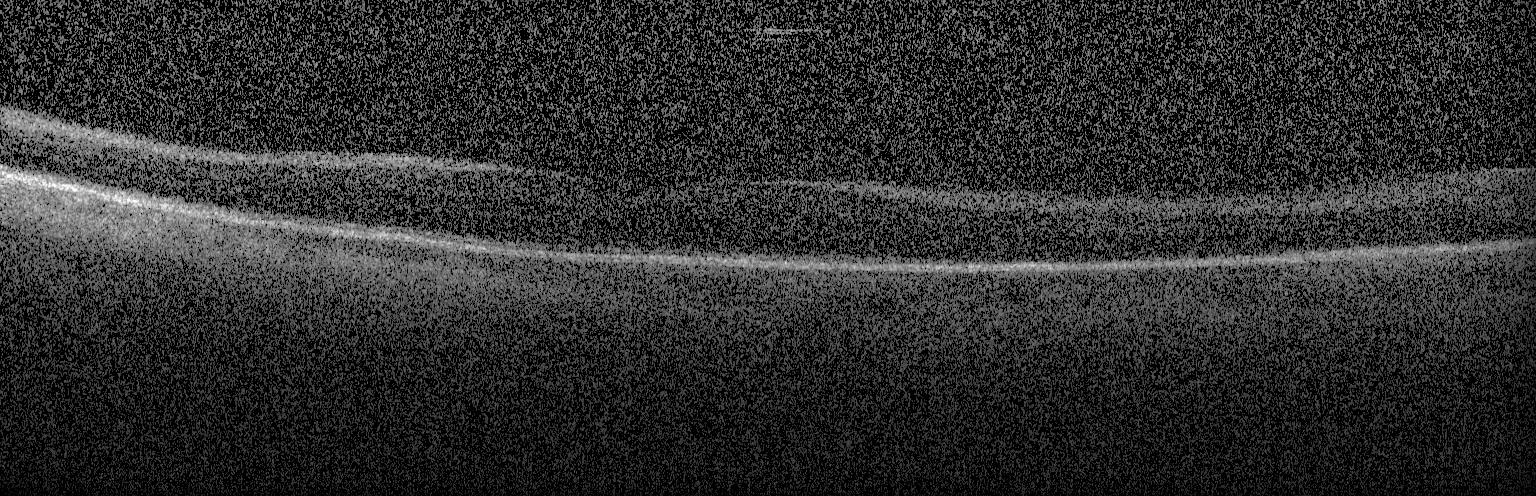 Optical coherence tomography B-scan. Macular scan. SD-OCT. Finding: neither CNV, DME, nor drusen.